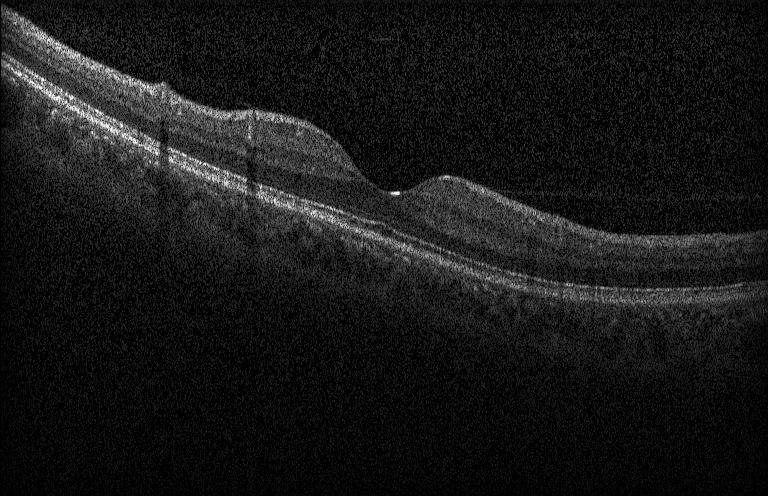 Retinal OCT cross-section
Diagnosis: no choroidal neovascularization, diabetic macular edema, or drusen.